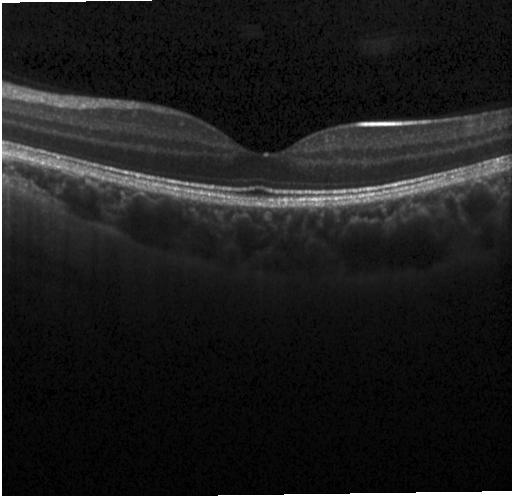 Spectral-domain OCT · fovea-centered · OCT B-scan — Diagnosis: no choroidal neovascularization, no diabetic macular edema, and no drusen.